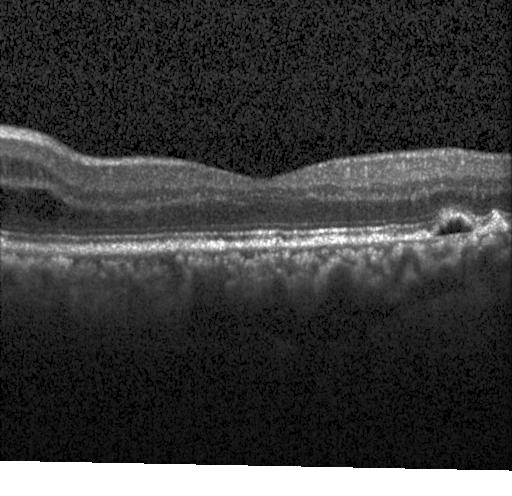
Macular scan; OCT B-scan; spectral-domain OCT — OCT finding: a choroidal neovascular membrane.